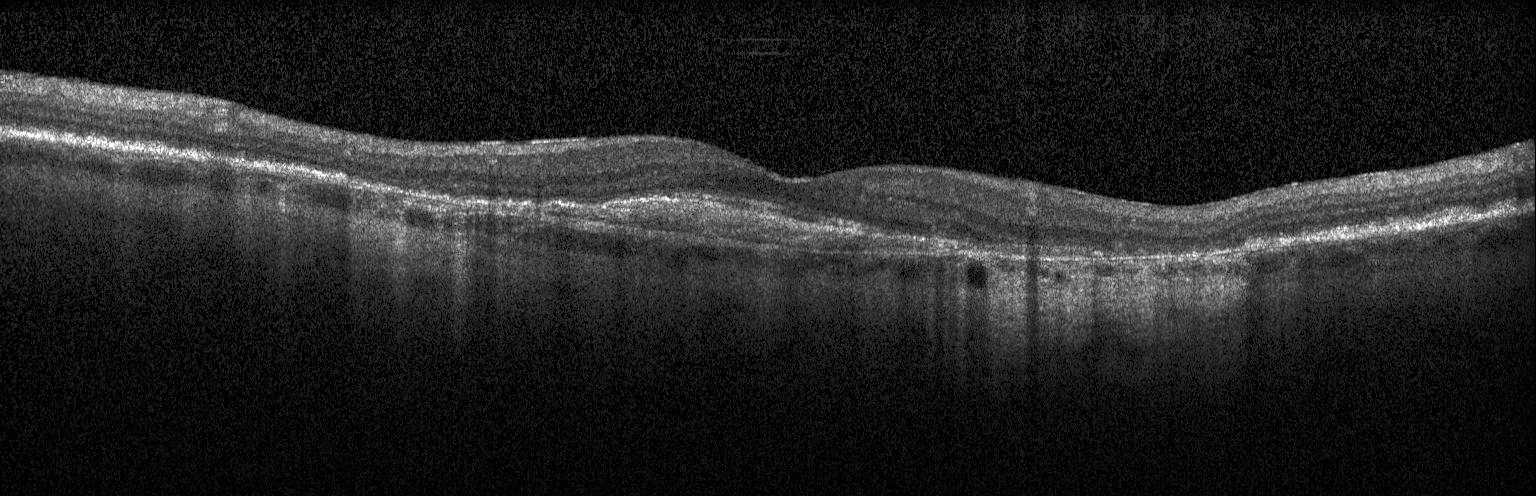

SD-OCT · Heidelberg Spectralis · optical coherence tomography scan.
Assessment: choroidal neovascularization (CNV).